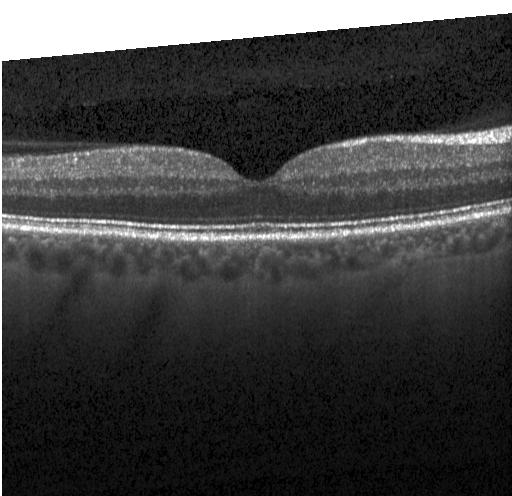

Through the macula. Optical coherence tomography B-scan — Impression: no choroidal neovascularization, no diabetic macular edema, and no drusen.